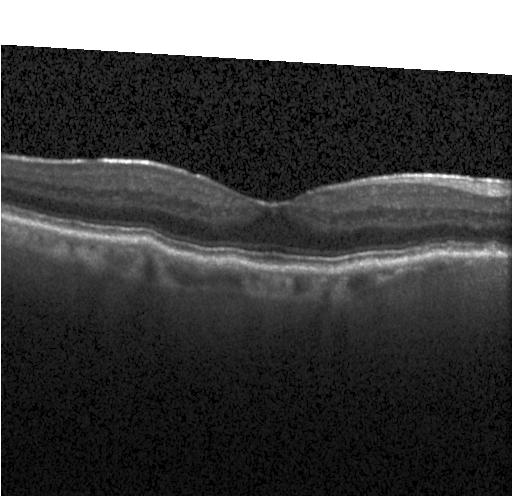
Retinal OCT cross-section, acquired on a Heidelberg Spectralis, macular scan, SD-OCT — This B-scan demonstrates drusen.